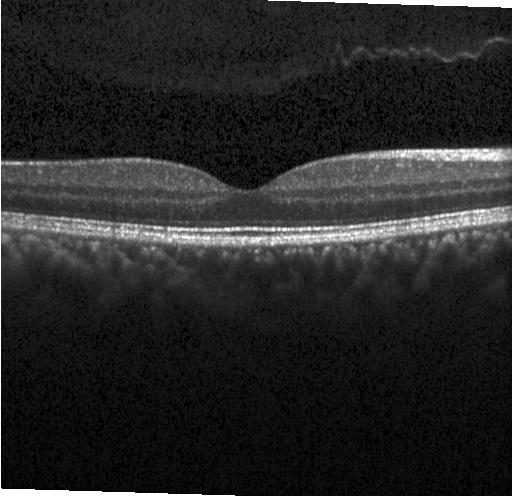 No evidence of choroidal neovascularization, diabetic macular edema, or drusen.